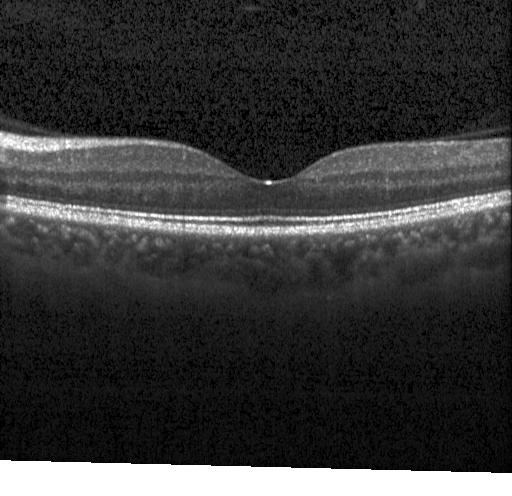 Horizontal scan through the fovea. Heidelberg Spectralis. Spectral-domain OCT. Optical coherence tomography B-scan.
Finding: no choroidal neovascularization, no diabetic macular edema, and no drusen.